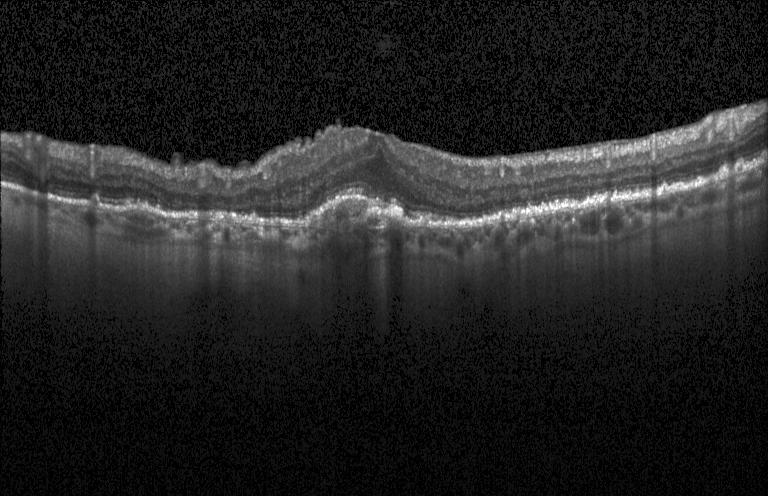
Retinal OCT B-scan; acquired on a Heidelberg Spectralis.
Assessment: a choroidal neovascular membrane.